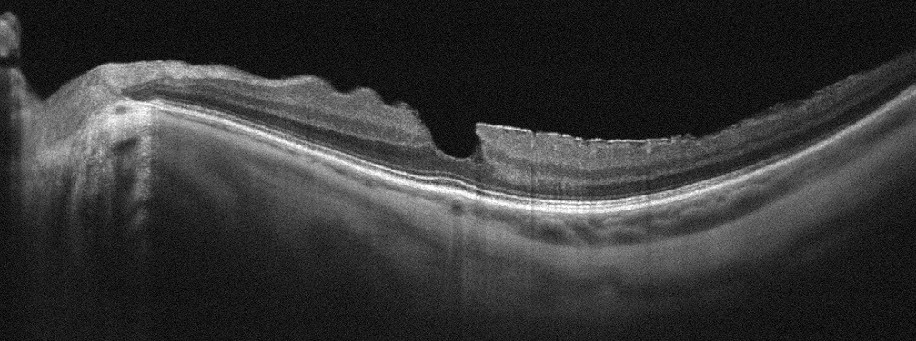

OCT B-scan. Through the macula.
Impression: ERM.